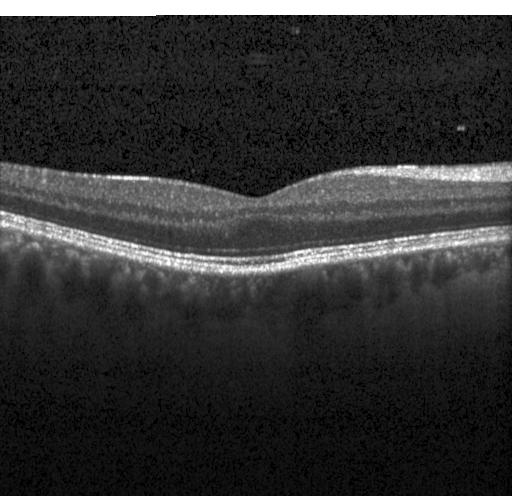 Retinal OCT B-scan. No evidence of choroidal neovascularization, diabetic macular edema, or drusen.